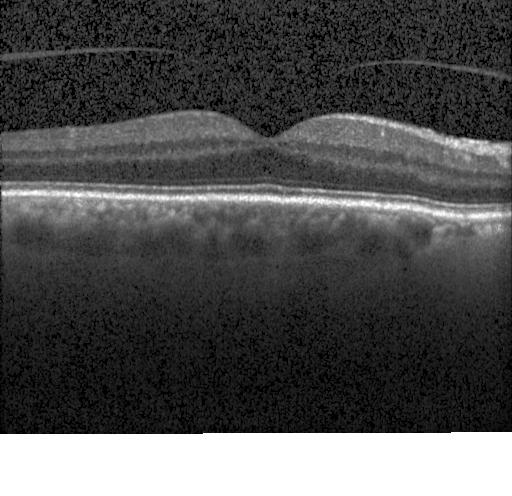

OCT B-scan; instrument: Heidelberg Spectralis
Assessment: neither choroidal neovascularization, diabetic macular edema, nor drusen.